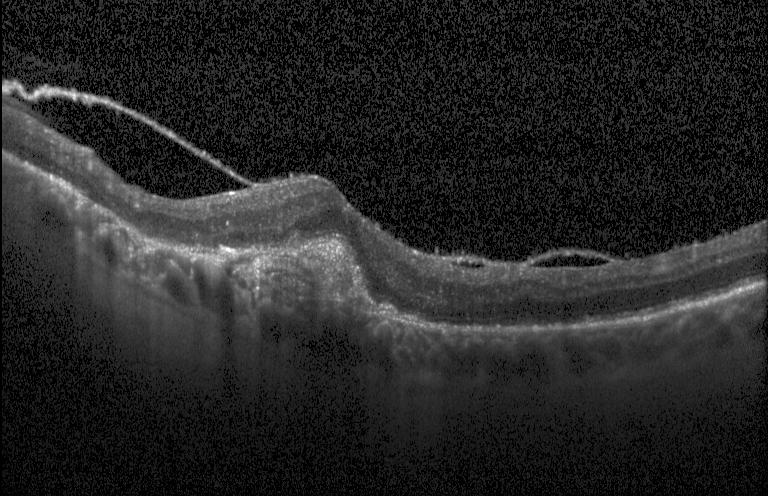 Optical coherence tomography scan. Spectral-domain optical coherence tomography. Instrument: Heidelberg Spectralis.
Macular OCT: a choroidal neovascular membrane.